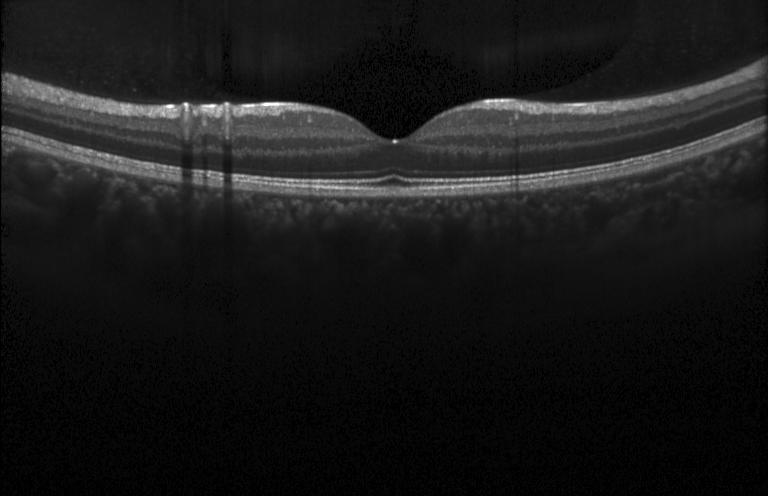 Diagnosis: neither CNV, DME, nor drusen.